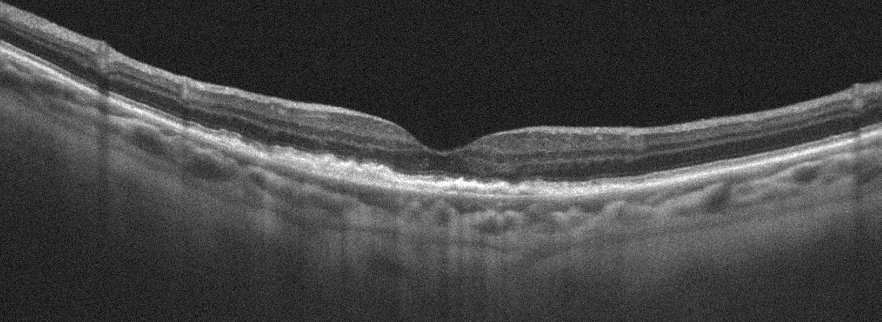

Oculus dexter, OCT B-scan. Age-related macular degeneration.